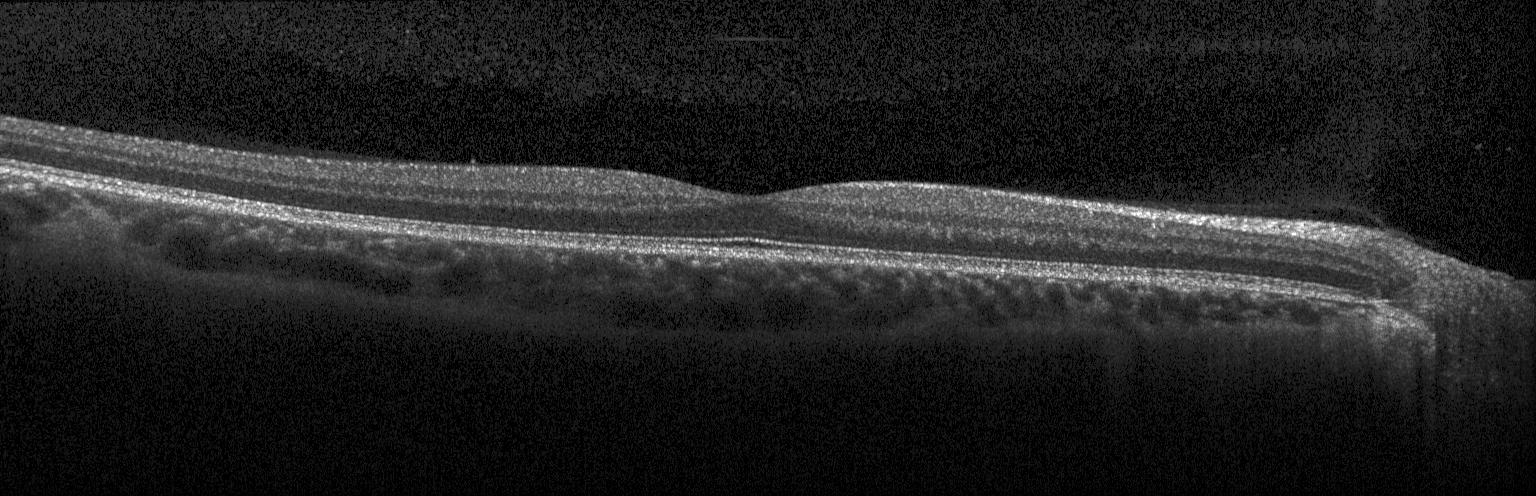

Optical coherence tomography B-scan — Neither CNV, DME, nor drusen.